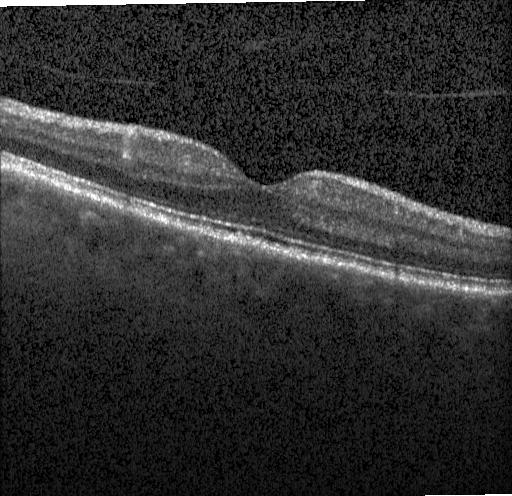
Heidelberg Spectralis OCT system; retinal OCT B-scan; fovea-centered. The scan shows no evidence of choroidal neovascularization, diabetic macular edema, or drusen.